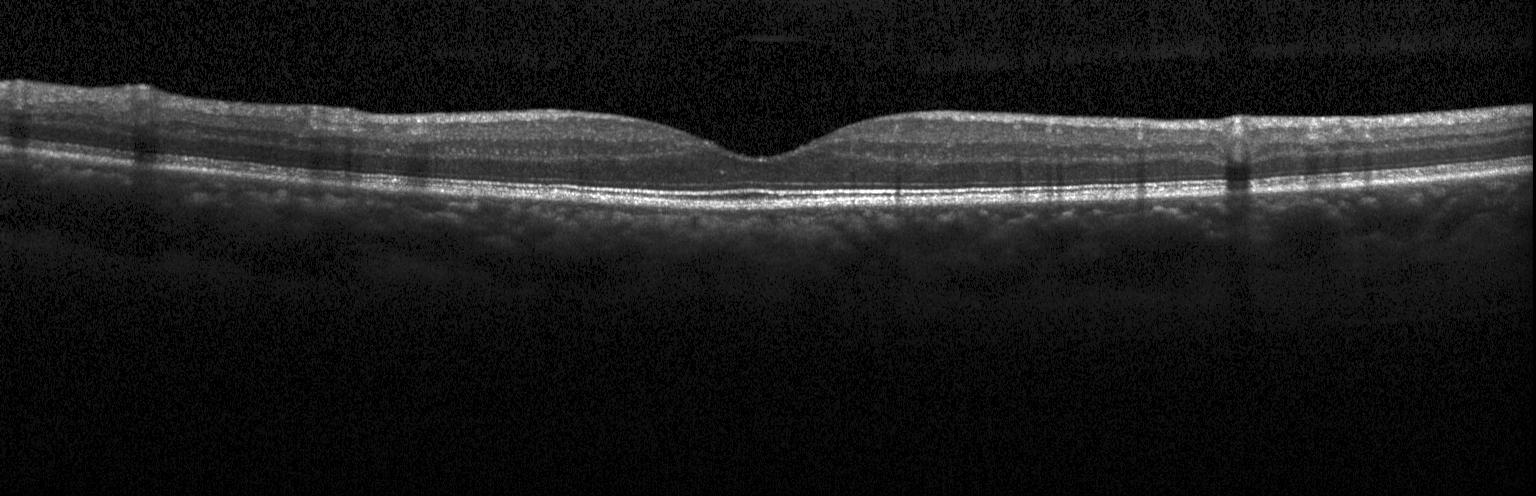

OCT B-scan showing neither CNV, DME, nor drusen.